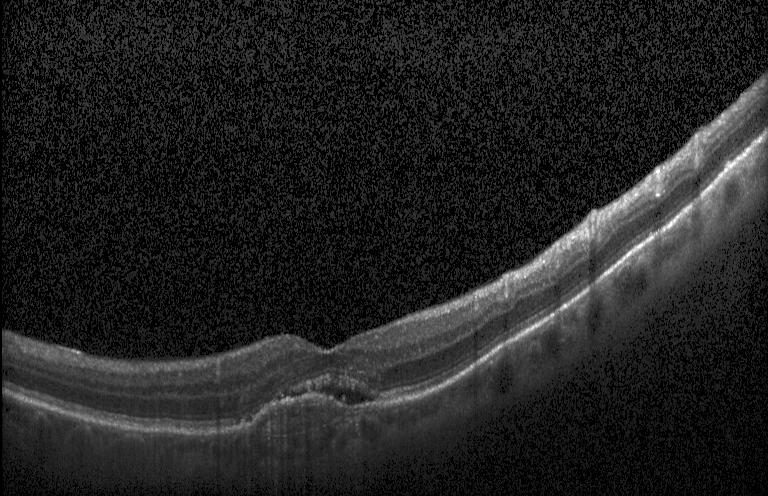

OCT B-scan
Finding: CNV.